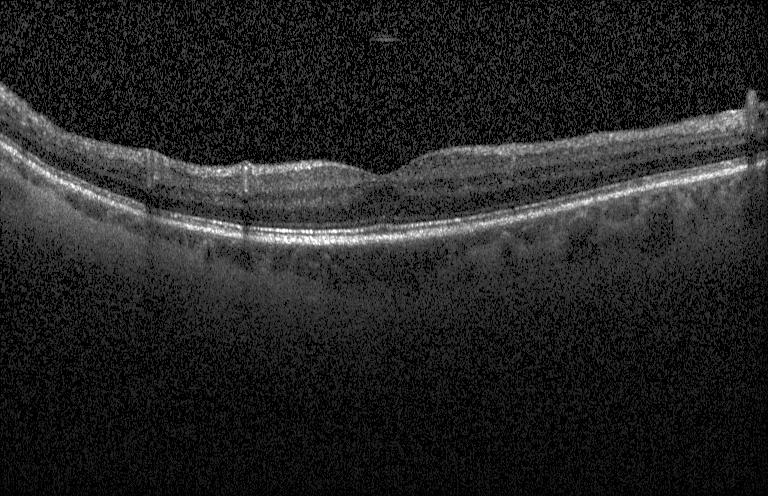

Through the macula, retinal OCT B-scan, Heidelberg Spectralis OCT system, spectral-domain optical coherence tomography
The scan shows neither choroidal neovascularization, diabetic macular edema, nor drusen.